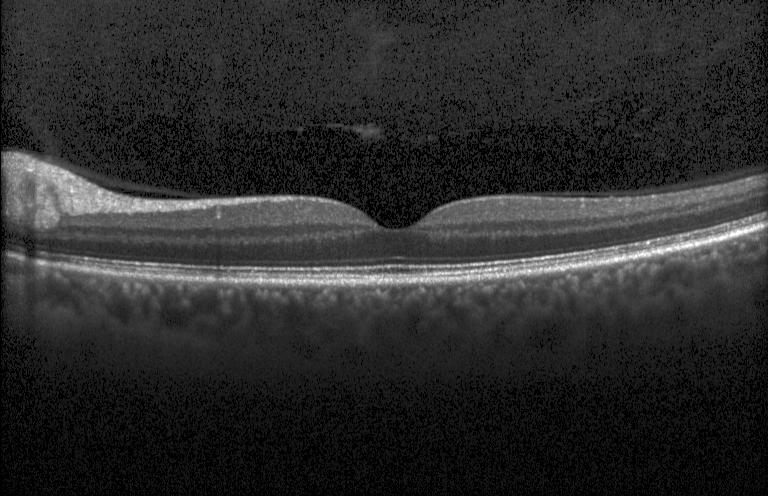

OCT B-scan, through the macula, instrument: Heidelberg Spectralis.
Dx: no evidence of choroidal neovascularization, diabetic macular edema, or drusen.